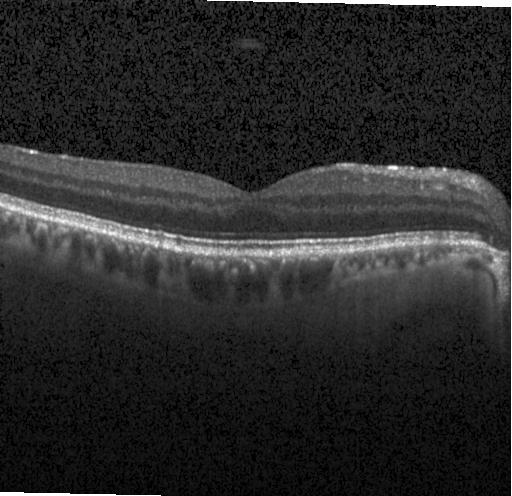
Retinal OCT B-scan; through the macula
Finding: no evidence of CNV, DME, or drusen.